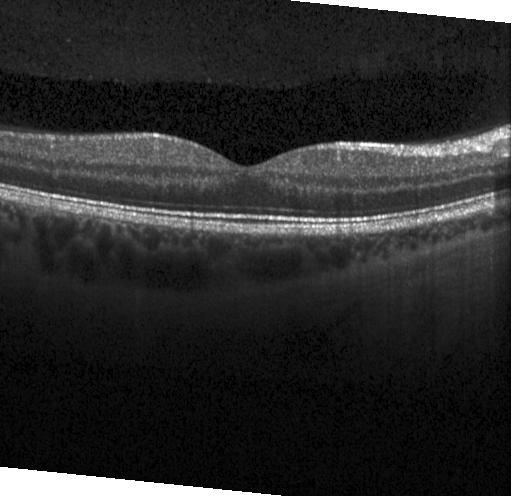
SD-OCT · OCT B-scan · instrument: Heidelberg Spectralis.
Assessment: no CNV, DME, or drusen.